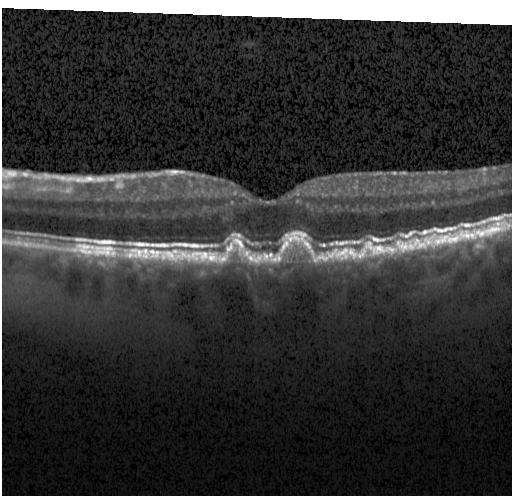
Dx: sub-RPE drusenoid deposits.